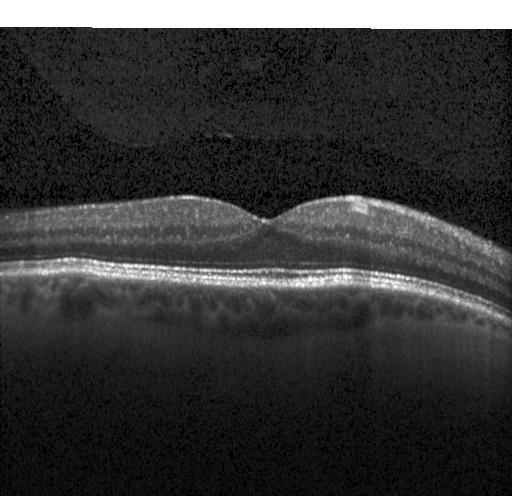 OCT B-scan. Finding: neither choroidal neovascularization, diabetic macular edema, nor drusen.